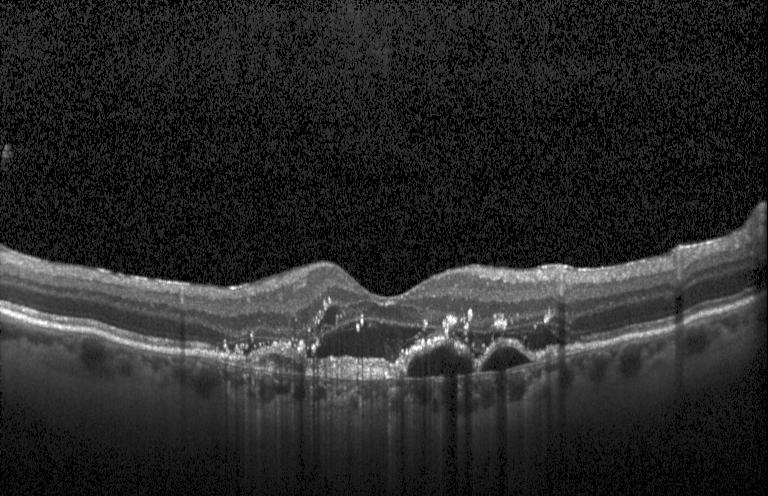
Spectral-domain optical coherence tomography; retinal OCT cross-section; acquired on a Heidelberg Spectralis; through the macula. This B-scan demonstrates a choroidal neovascular membrane.